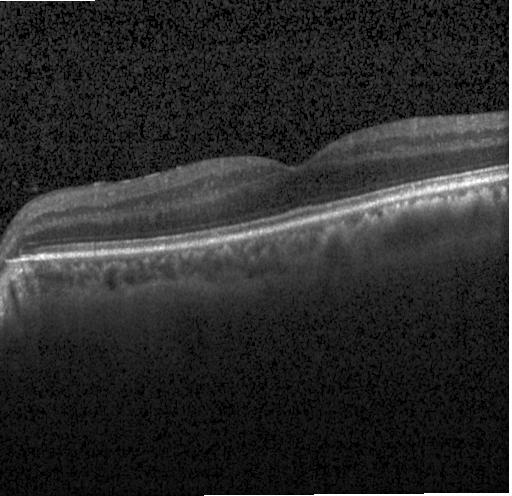
Retinal OCT B-scan · macular scan — The scan shows no choroidal neovascularization, no diabetic macular edema, and no drusen.